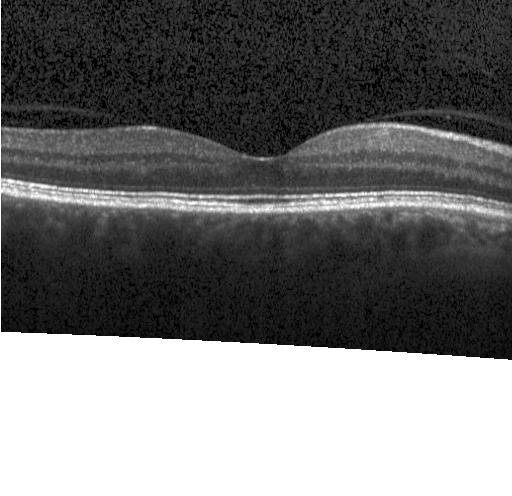 No evidence of CNV, DME, or drusen.